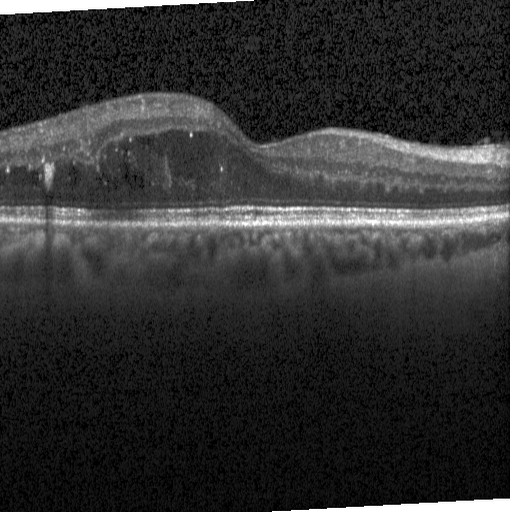

Spectral-domain optical coherence tomography; horizontal scan through the fovea; optical coherence tomography B-scan; instrument: Heidelberg Spectralis. The scan shows diabetic macular edema.